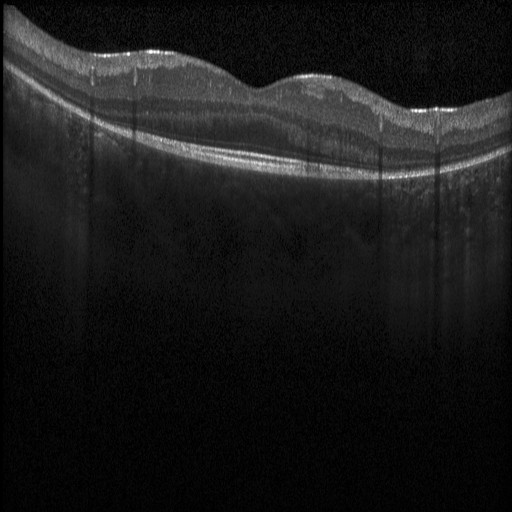

OCT B-scan; spectral-domain OCT.
Assessment: diabetic macular edema.